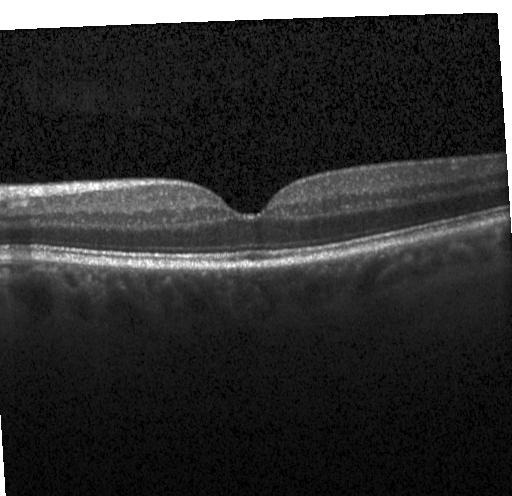

Spectral-domain OCT · OCT line scan · acquired on a Heidelberg Spectralis.
This B-scan demonstrates neither choroidal neovascularization, diabetic macular edema, nor drusen.